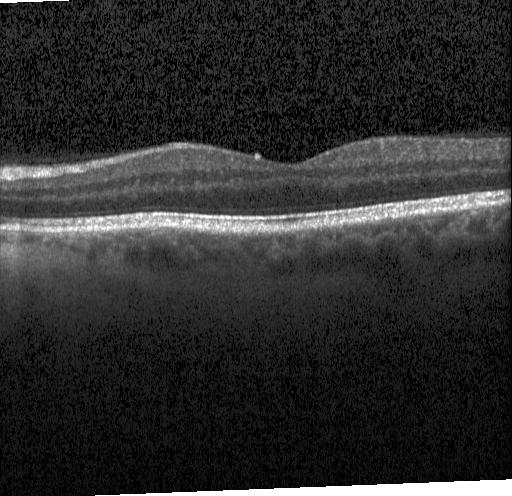
Heidelberg Spectralis OCT system · retinal OCT B-scan — Macular OCT: no evidence of choroidal neovascularization, diabetic macular edema, or drusen.